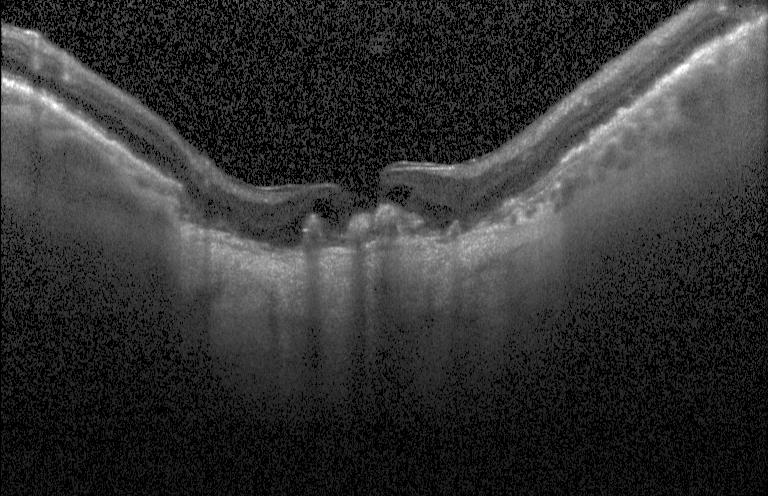 Optical coherence tomography B-scan — OCT finding: a choroidal neovascular membrane.